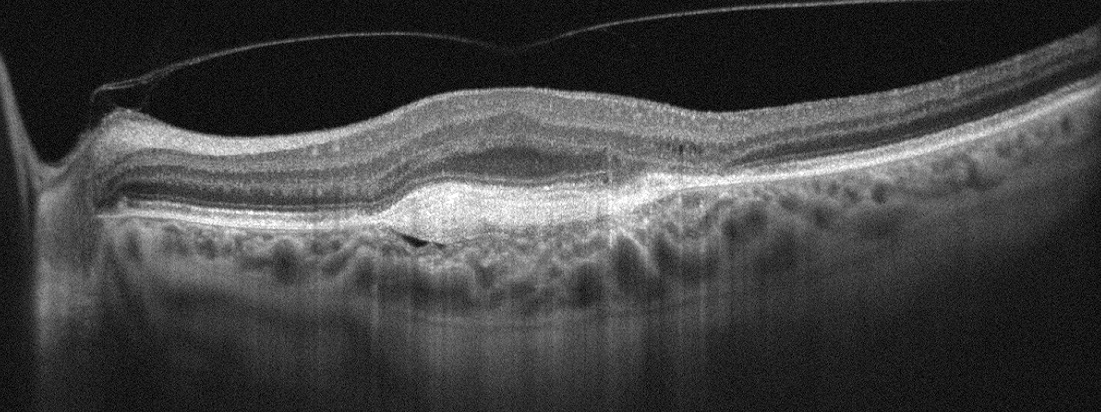
Dx: AMD.